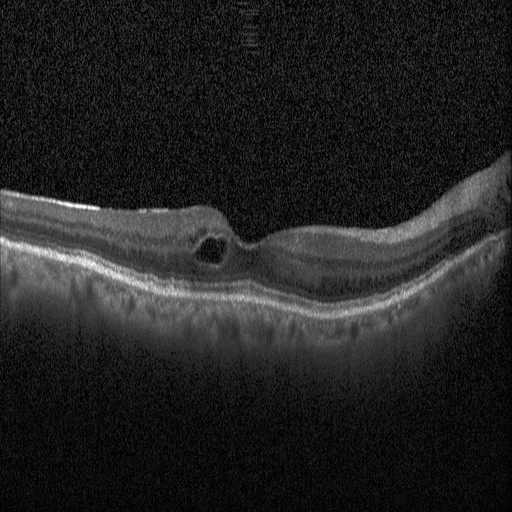 Spectral-domain optical coherence tomography, optical coherence tomography B-scan, through the macula, Heidelberg Spectralis OCT system. Dx: DME.